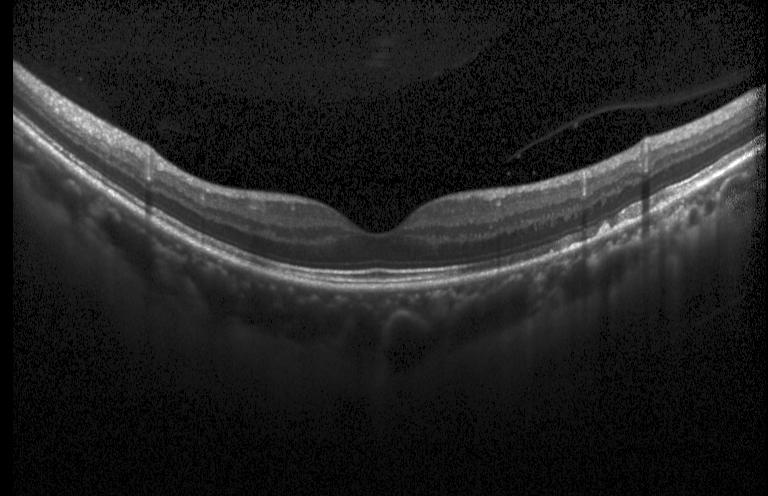 Spectral-domain optical coherence tomography · retinal OCT cross-section.
Macular OCT: multiple drusen.